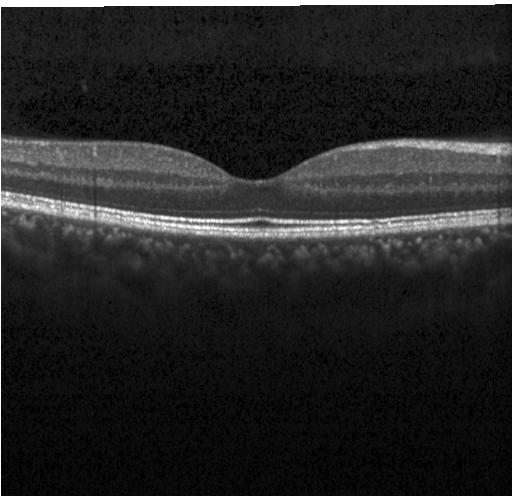

OCT line scan. Impression: no evidence of choroidal neovascularization, diabetic macular edema, or drusen.